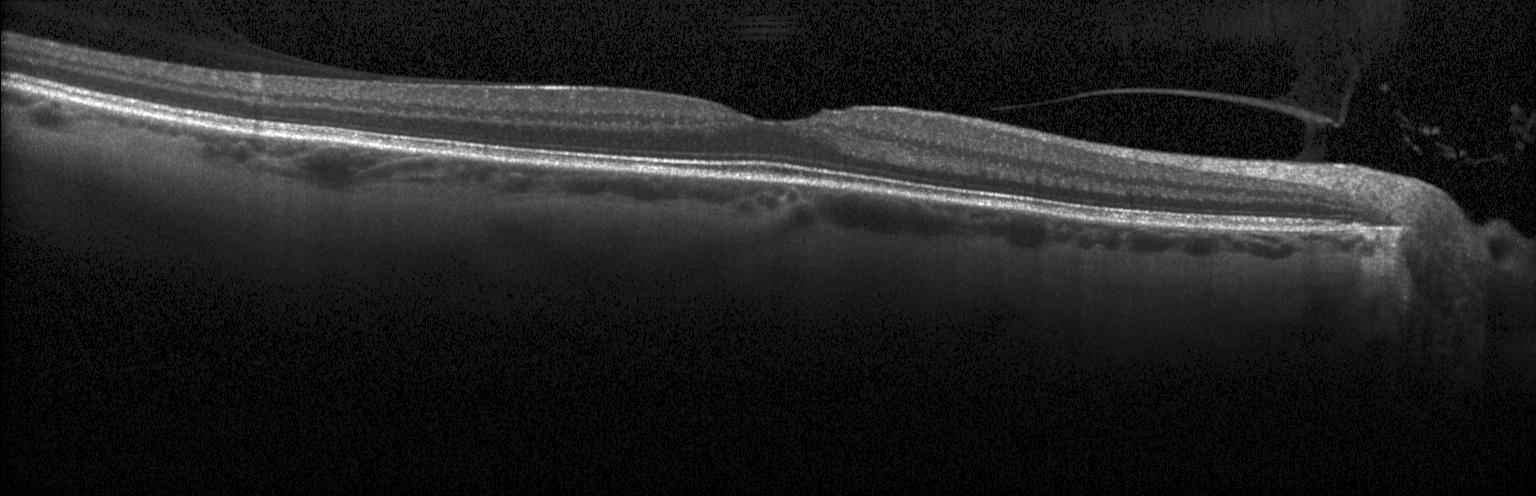
Acquired on a Heidelberg Spectralis. OCT line scan. Assessment: no choroidal neovascularization, diabetic macular edema, or drusen.